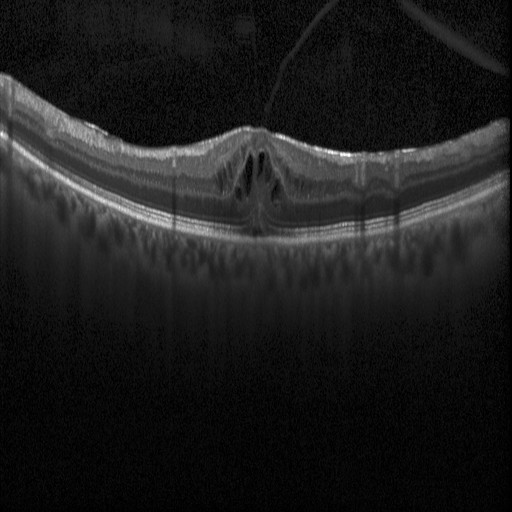 Diagnosis: DME.